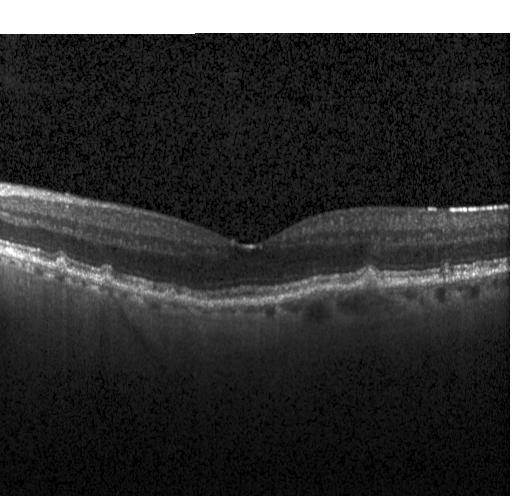
Retinal OCT cross-section, fovea-centered.
Impression: multiple drusen.